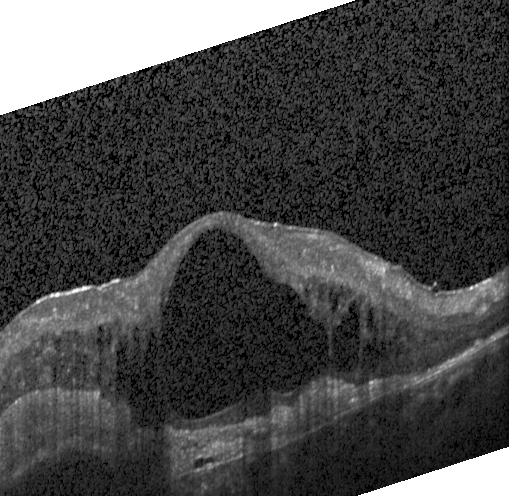

Retinal OCT cross-section, centered on the fovea.
This B-scan demonstrates CNV.